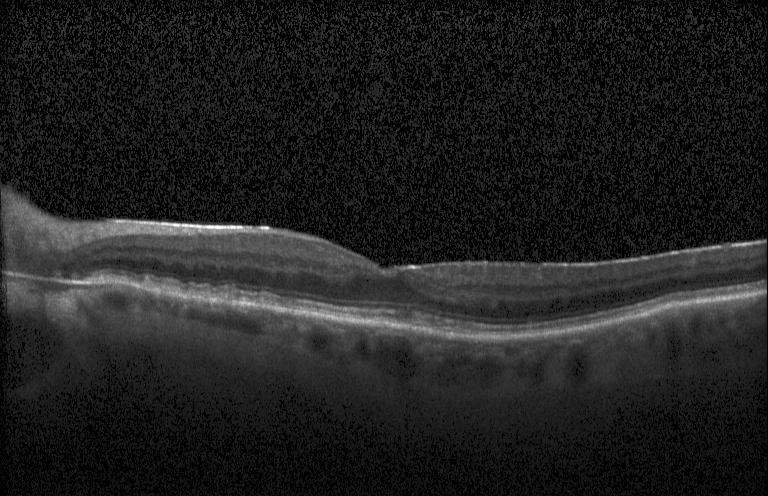 OCT B-scan. Heidelberg Spectralis OCT system.
Drusen.